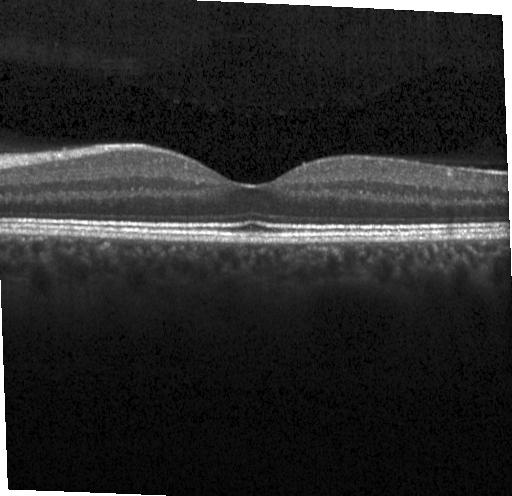
Spectral-domain OCT, optical coherence tomography B-scan
Impression: no evidence of CNV, DME, or drusen.